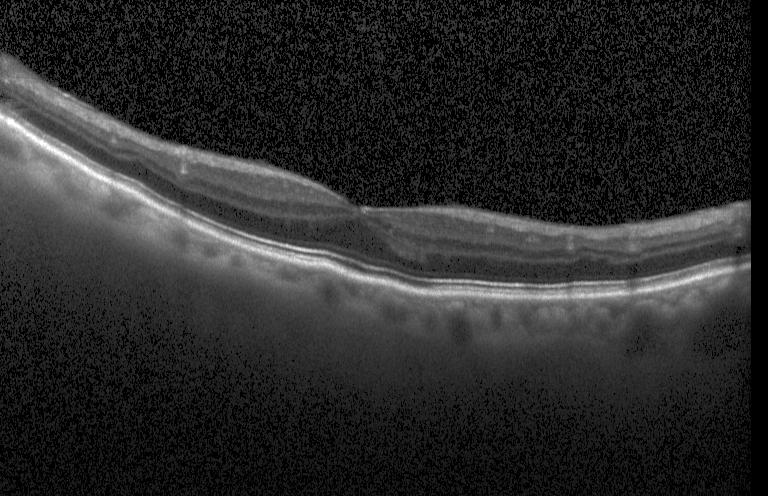

Optical coherence tomography scan.
Dx: no CNV, no DME, and no drusen.